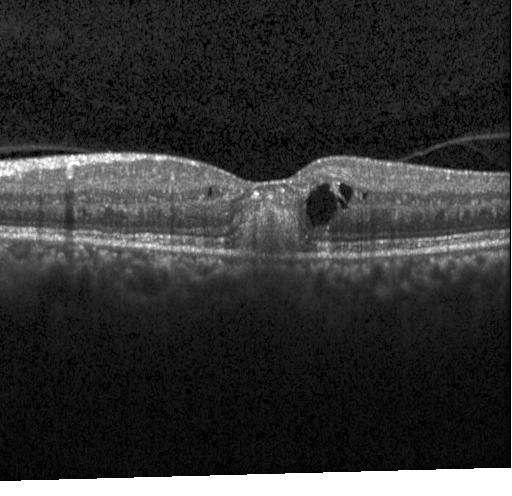
Optical coherence tomography B-scan
OCT finding: choroidal neovascularization.